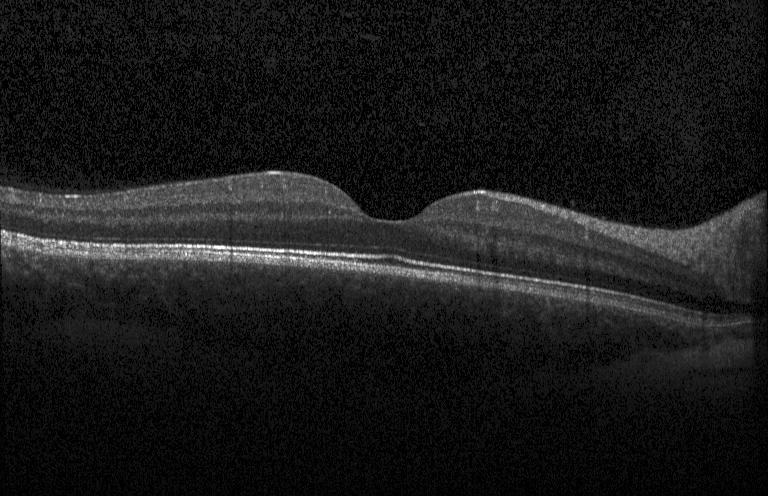

Horizontal scan through the fovea · OCT line scan · SD-OCT. Dx: no choroidal neovascularization, diabetic macular edema, or drusen.